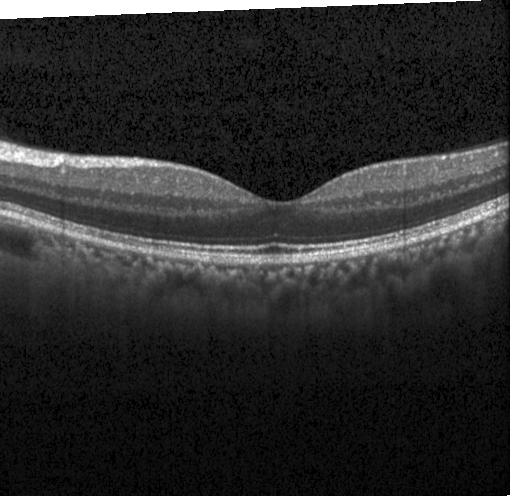

Impression: neither choroidal neovascularization, diabetic macular edema, nor drusen.